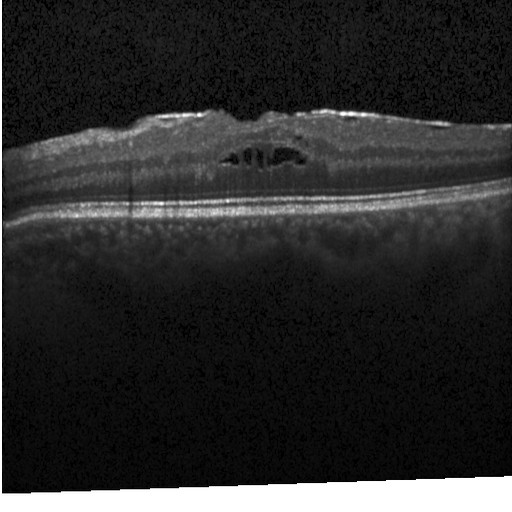

Spectral-domain optical coherence tomography. Optical coherence tomography B-scan. Through the macula
Impression: diabetic macular edema.